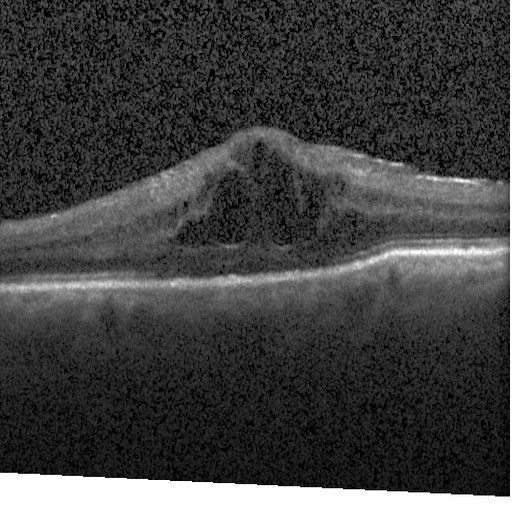
OCT line scan · Heidelberg Spectralis.
Impression: diabetic macular edema.